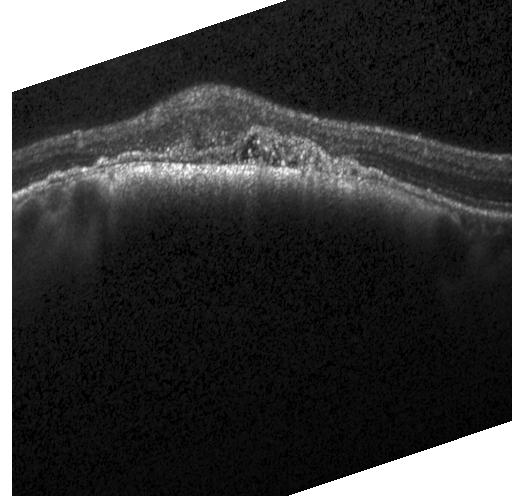
Heidelberg Spectralis OCT system, retinal OCT cross-section
Finding: a choroidal neovascular membrane.